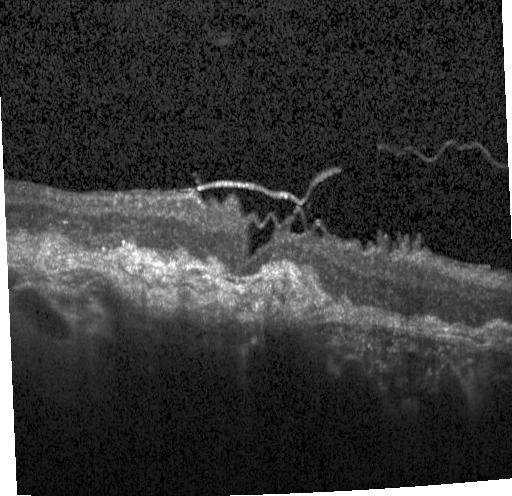 The scan shows a choroidal neovascular membrane.